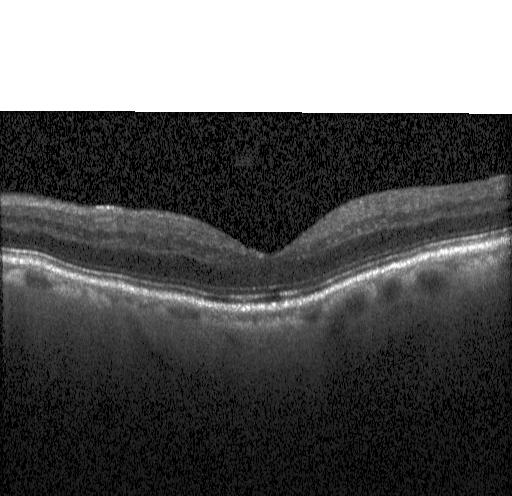

Optical coherence tomography B-scan. Diagnosis: no evidence of choroidal neovascularization, diabetic macular edema, or drusen.